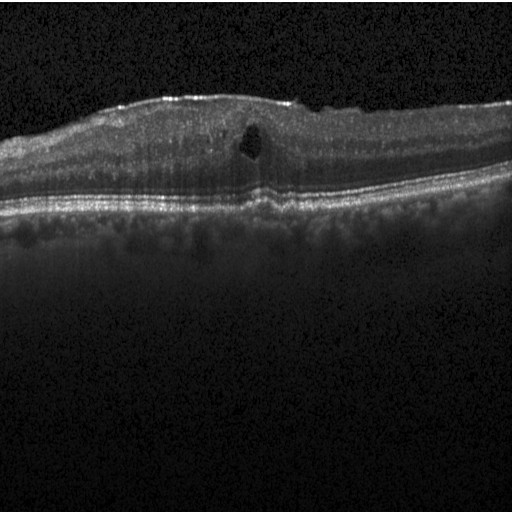

SD-OCT · acquired on a Heidelberg Spectralis · retinal OCT cross-section. Finding: diabetic macular edema.